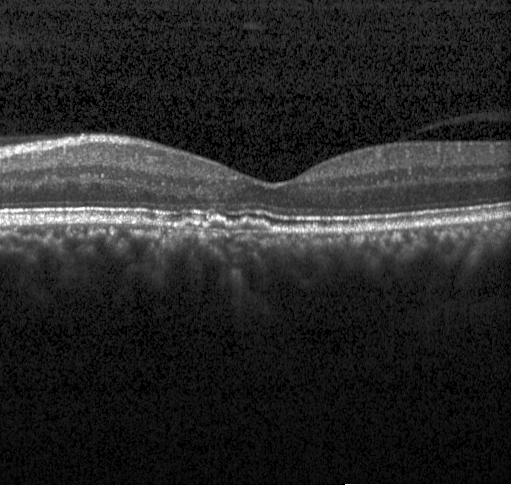

Spectral-domain OCT, optical coherence tomography B-scan, centered on the fovea — Assessment: multiple drusen.